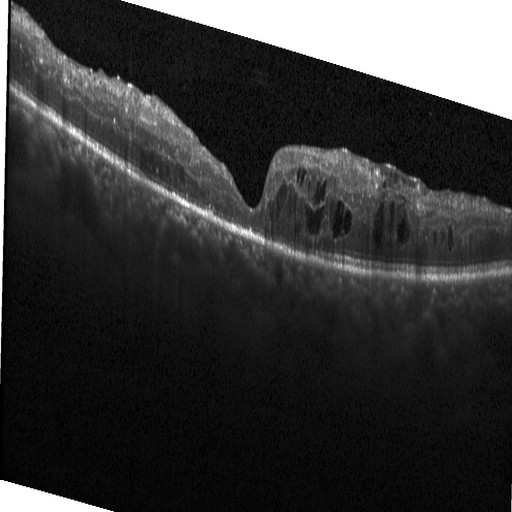 Retinal OCT B-scan; spectral-domain OCT; Heidelberg Spectralis OCT system. OCT finding: diabetic macular edema (DME).